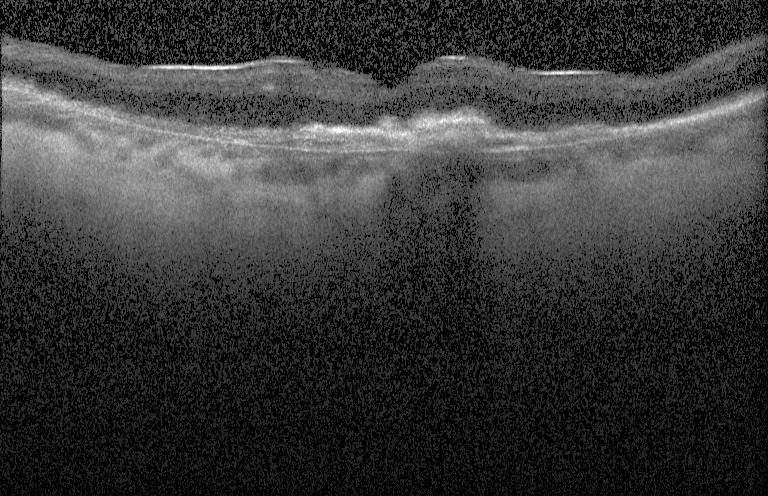
The scan shows choroidal neovascularization.